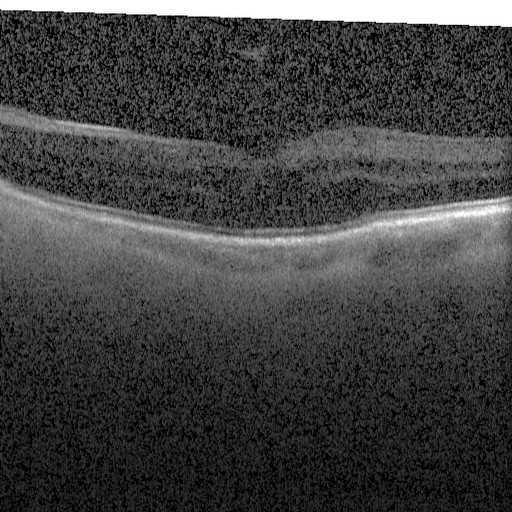

Centered on the fovea, spectral-domain OCT, OCT B-scan.
Macular OCT: diabetic macular edema (DME).